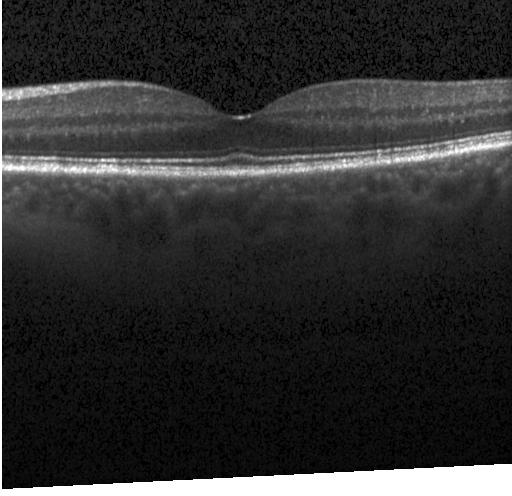
No choroidal neovascularization, no diabetic macular edema, and no drusen.